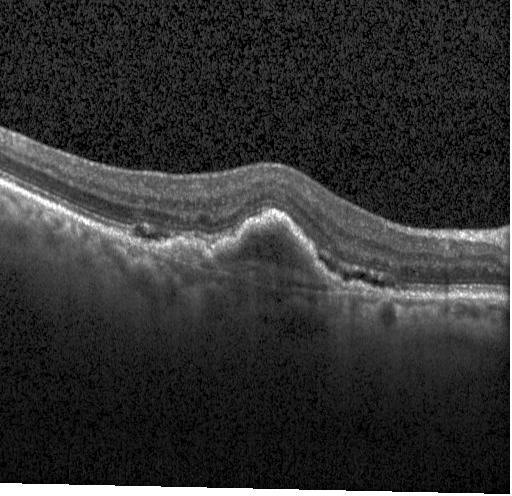 Through the macula; retinal OCT cross-section; SD-OCT — The scan shows a choroidal neovascular membrane.